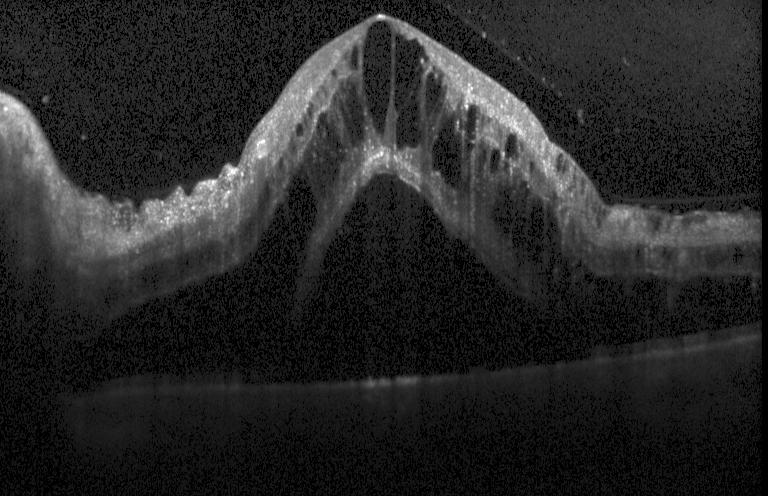 Heidelberg Spectralis · retinal OCT cross-section. Diabetic macular edema.